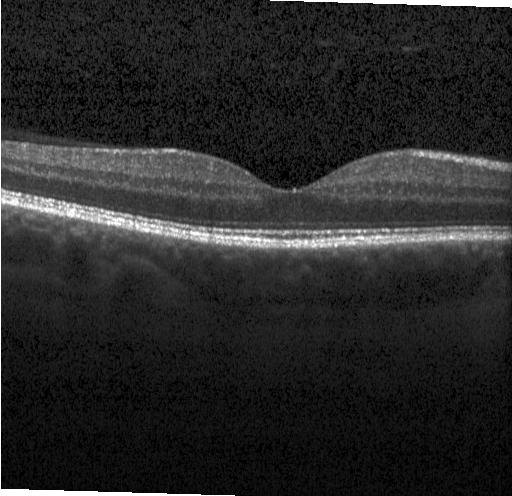 The scan shows no evidence of CNV, DME, or drusen.